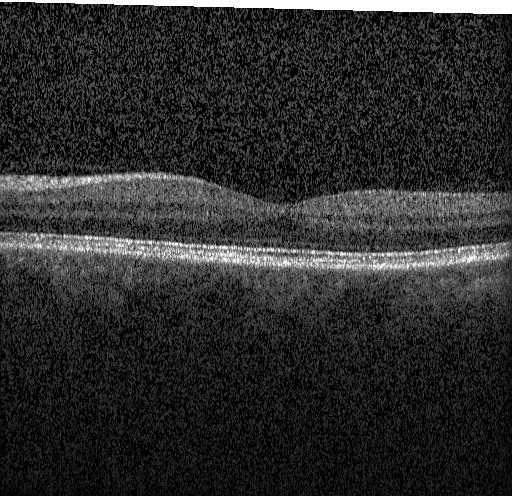

Fovea-centered. Spectral-domain OCT. Heidelberg Spectralis OCT system. Retinal OCT B-scan
Finding: no evidence of CNV, DME, or drusen.